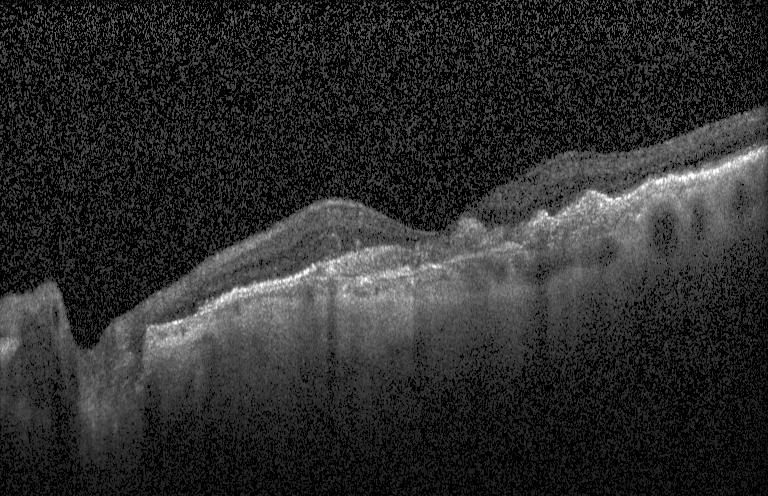 Assessment: a choroidal neovascular membrane.